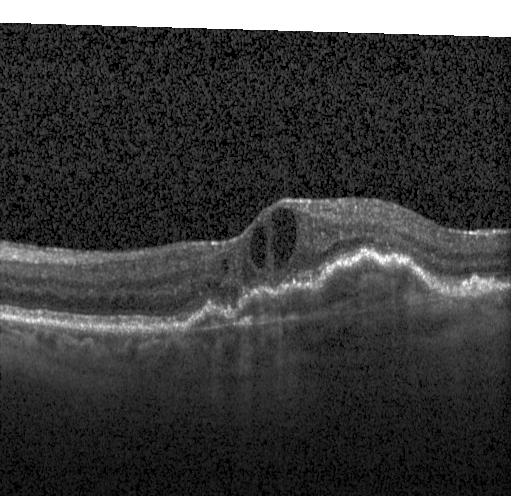
Through the macula · retinal OCT cross-section · spectral-domain OCT — Assessment: choroidal neovascularization (CNV).